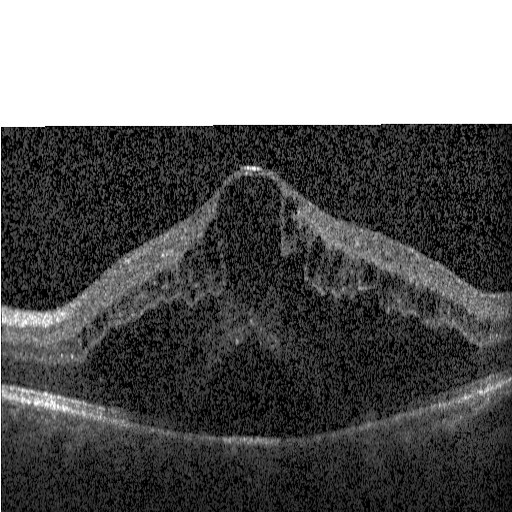 Optical coherence tomography scan · spectral-domain optical coherence tomography · Heidelberg Spectralis · centered on the fovea
Assessment: diabetic macular edema.